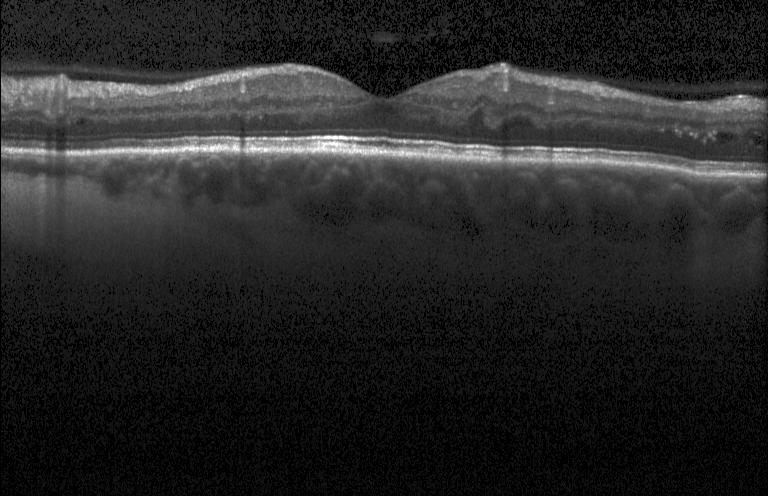

SD-OCT; OCT B-scan. This B-scan demonstrates diabetic macular edema (DME).